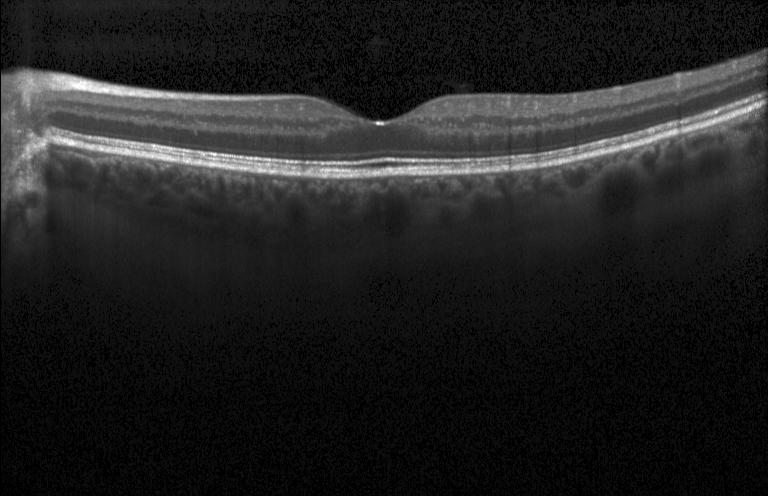
Optical coherence tomography scan · fovea-centered · spectral-domain optical coherence tomography — Impression: no evidence of CNV, DME, or drusen.